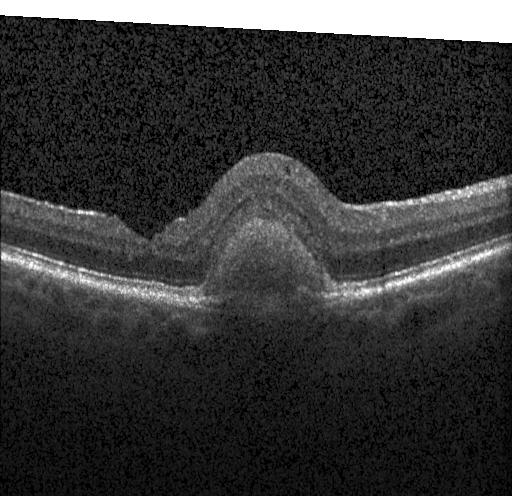
Through the macula, acquired on a Heidelberg Spectralis, spectral-domain optical coherence tomography, optical coherence tomography scan.
Diagnosis: a choroidal neovascular membrane.